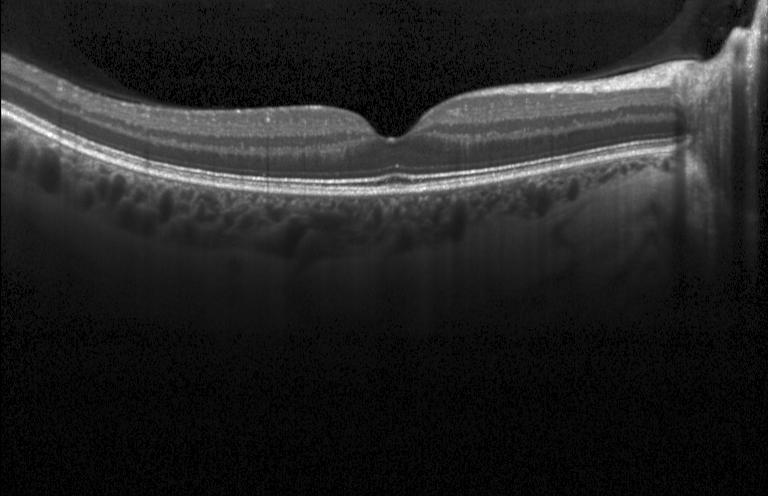
Optical coherence tomography scan · centered on the fovea.
Diagnosis: no choroidal neovascularization, diabetic macular edema, or drusen.